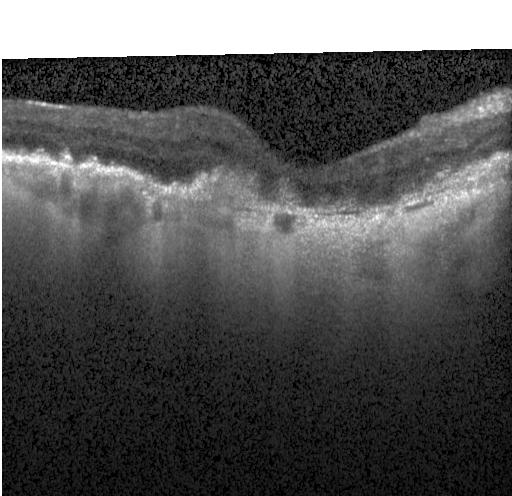

Macular OCT: a choroidal neovascular membrane.